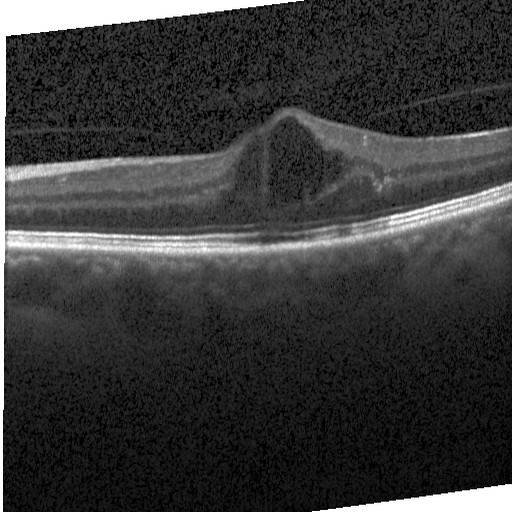

Finding: diabetic macular edema (DME).